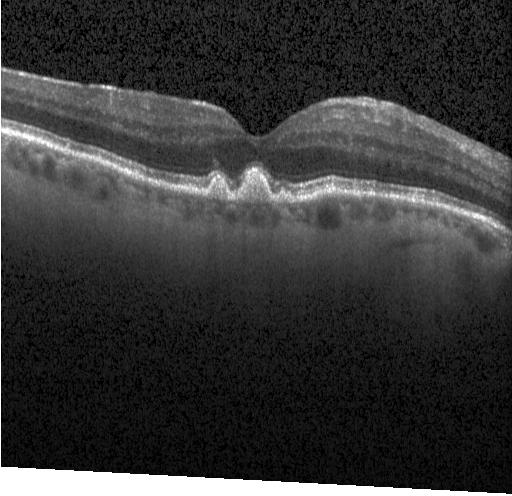
Macular OCT: drusen.